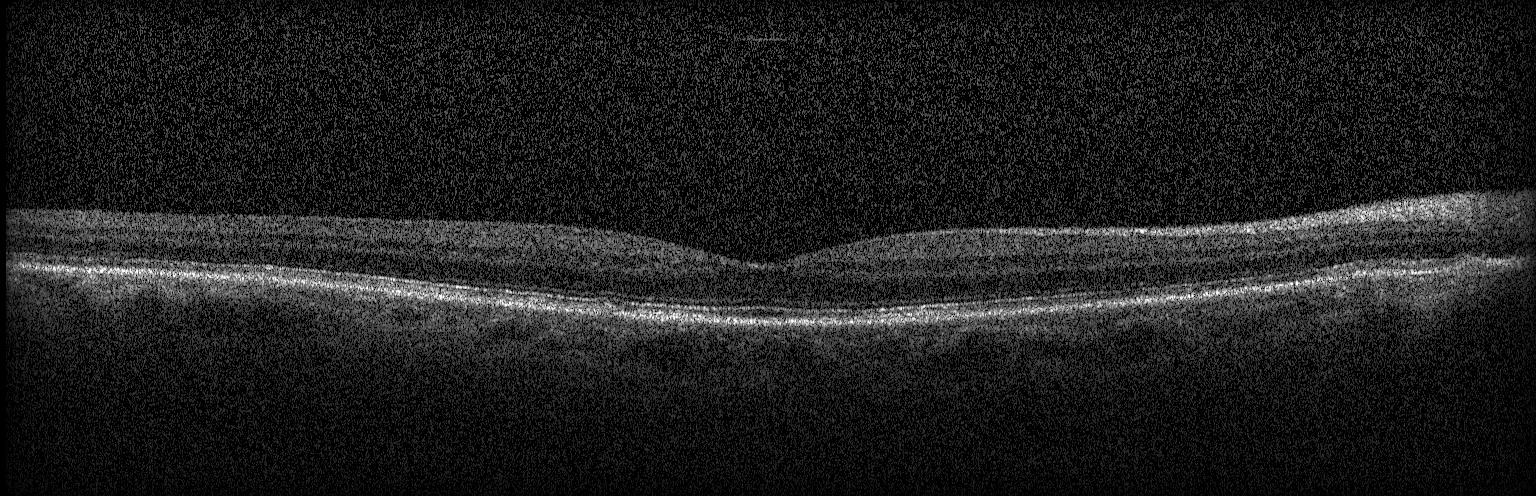

Spectral-domain OCT; Heidelberg Spectralis OCT system; OCT B-scan; centered on the fovea — Impression: no choroidal neovascularization, diabetic macular edema, or drusen.